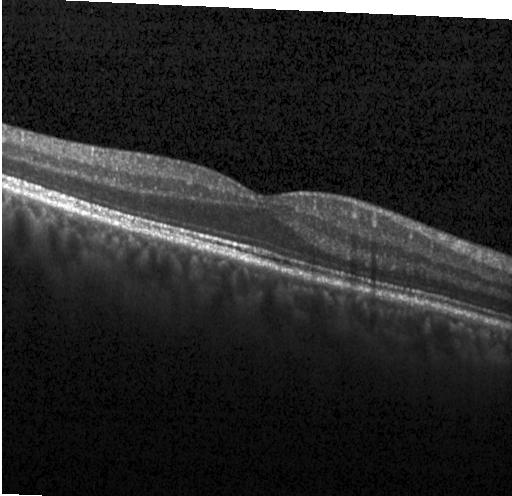
Spectral-domain optical coherence tomography; macular scan; OCT B-scan
Diagnosis: neither choroidal neovascularization, diabetic macular edema, nor drusen.